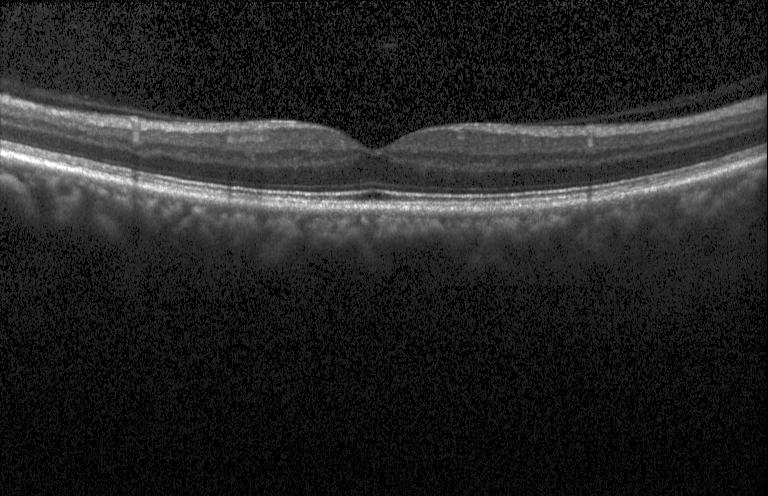
Optical coherence tomography scan.
Assessment: no evidence of choroidal neovascularization, diabetic macular edema, or drusen.